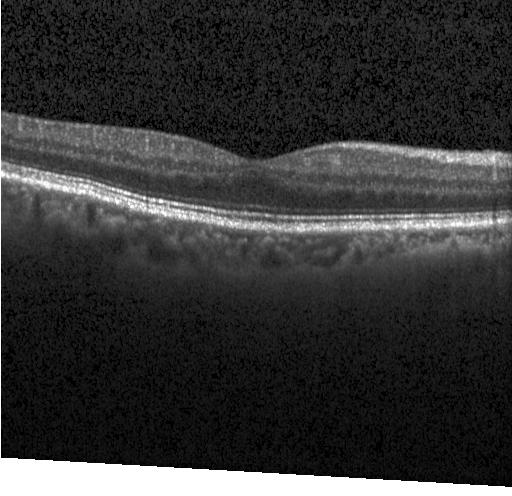 OCT line scan — Assessment: neither choroidal neovascularization, diabetic macular edema, nor drusen.